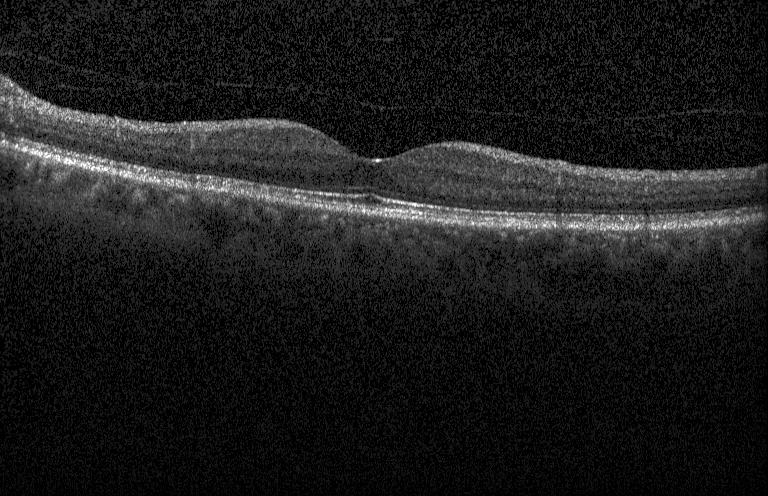

OCT B-scan — Impression: no evidence of choroidal neovascularization, diabetic macular edema, or drusen.